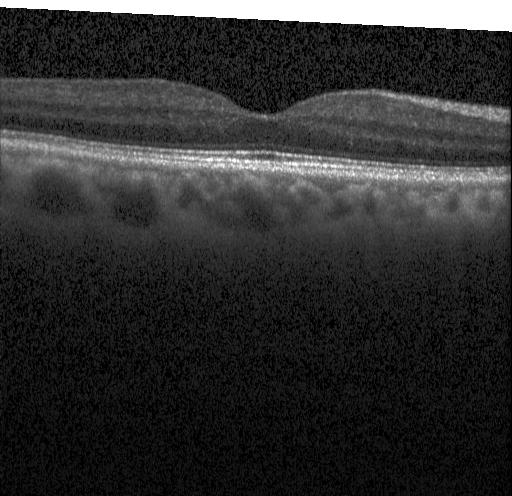
Centered on the fovea · retinal OCT B-scan — The scan shows no choroidal neovascularization, diabetic macular edema, or drusen.